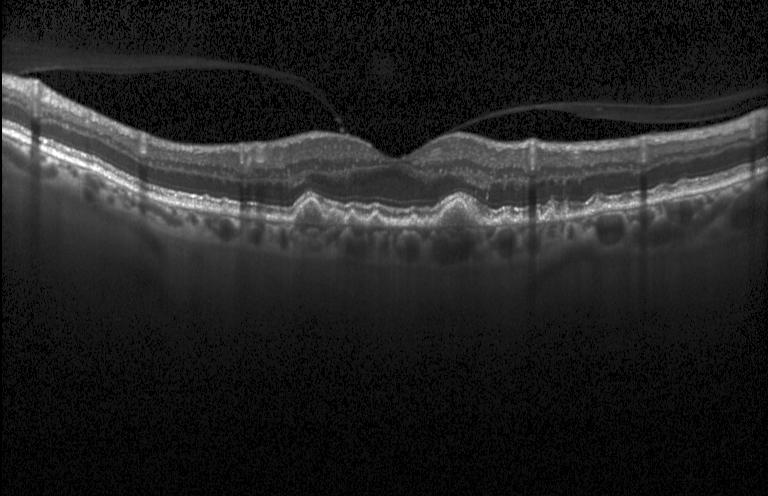

Retinal OCT cross-section showing sub-RPE drusenoid deposits.